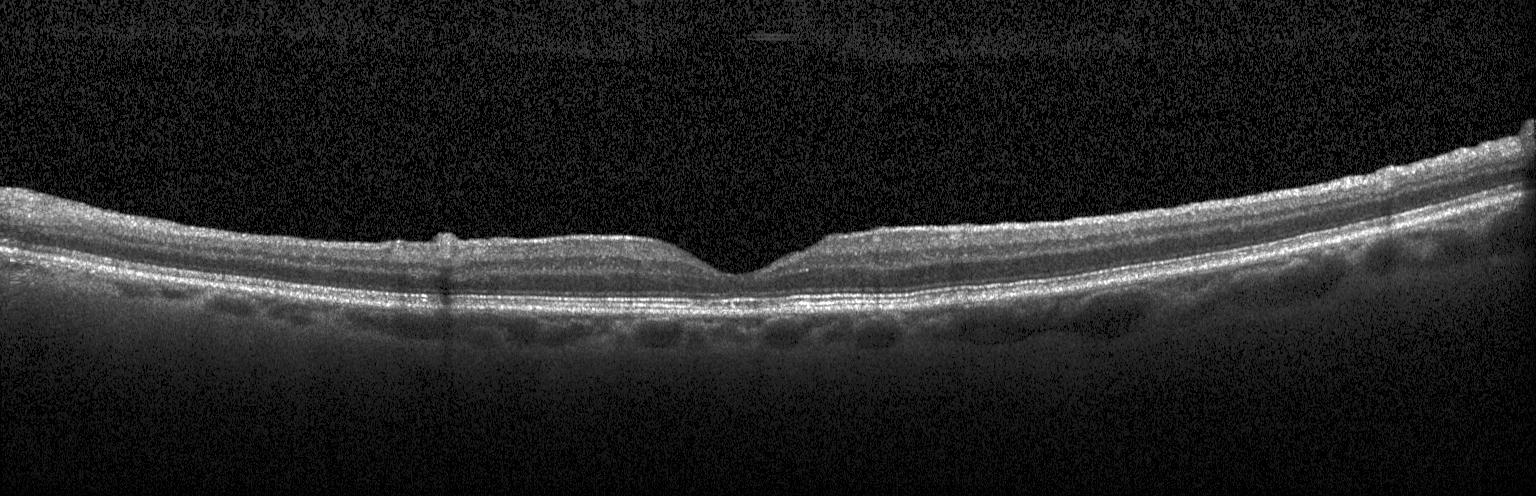

Instrument: Heidelberg Spectralis, SD-OCT, OCT line scan
Finding: no evidence of CNV, DME, or drusen.